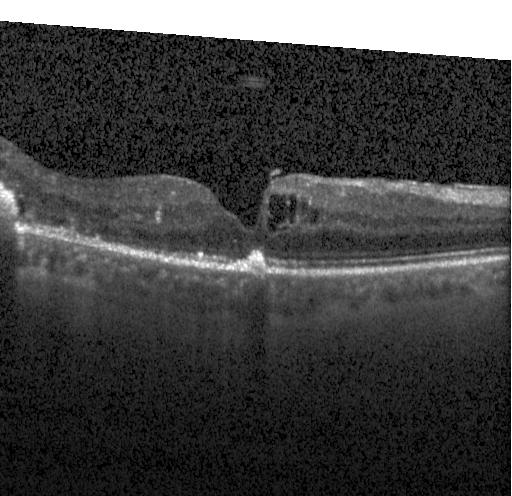

Optical coherence tomography scan · Heidelberg Spectralis OCT system · macular scan · spectral-domain optical coherence tomography. Finding: choroidal neovascularization.